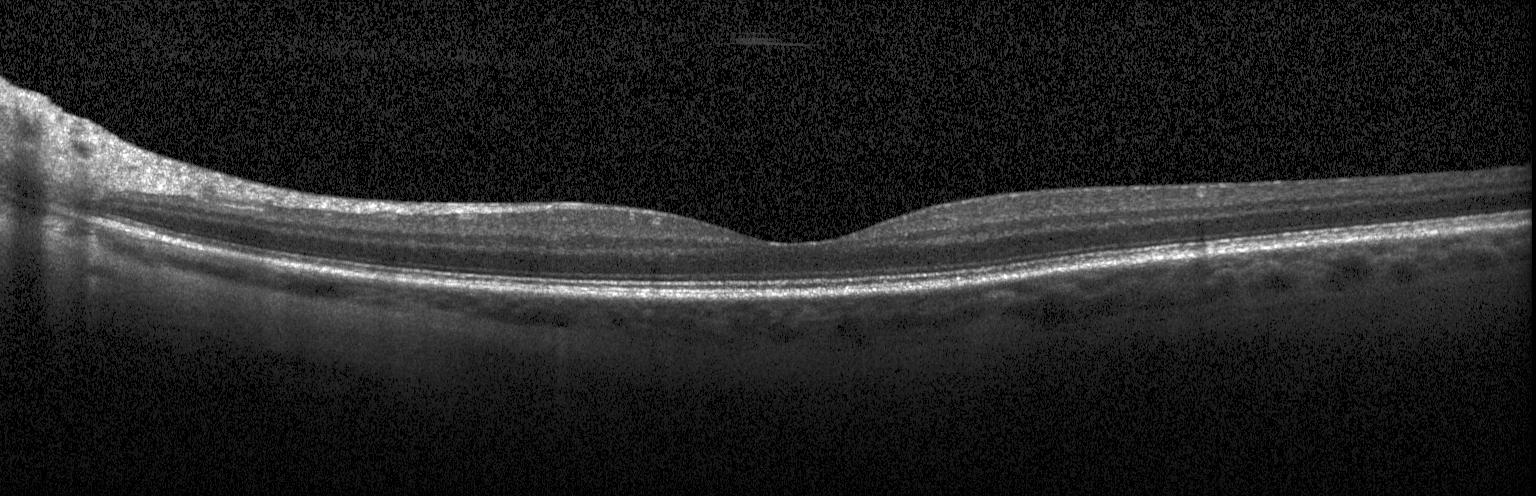 Retinal OCT B-scan — Diagnosis: no choroidal neovascularization, diabetic macular edema, or drusen.